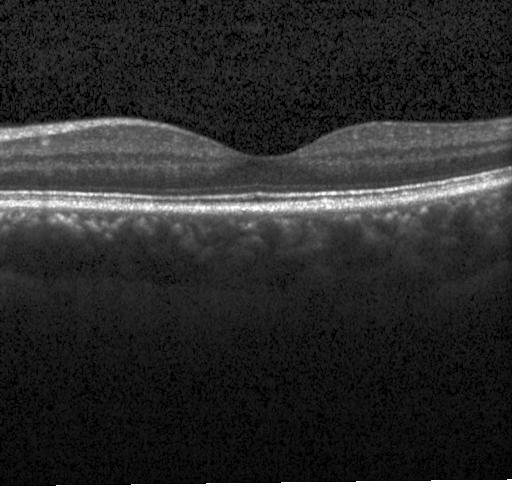 Diagnosis: neither choroidal neovascularization, diabetic macular edema, nor drusen.